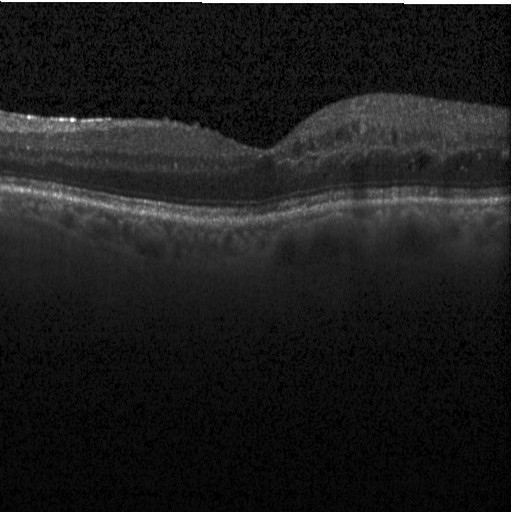
Macular scan · SD-OCT · instrument: Heidelberg Spectralis · optical coherence tomography B-scan
Diabetic macular edema.